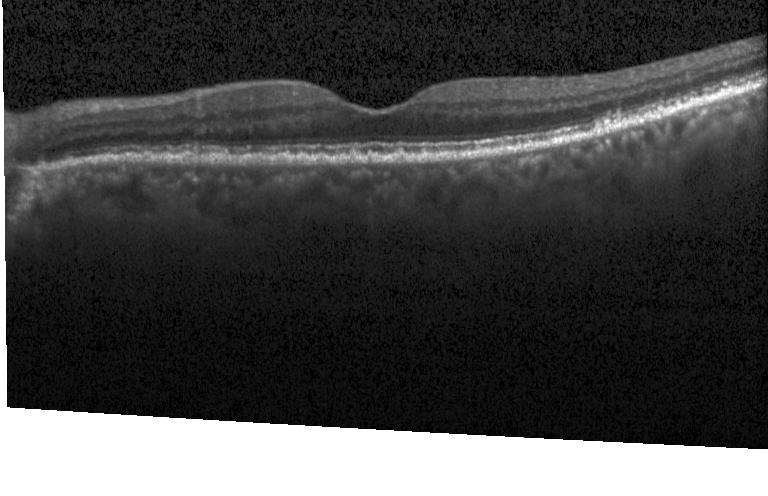
Retinal OCT cross-section — Impression: sub-RPE drusenoid deposits.